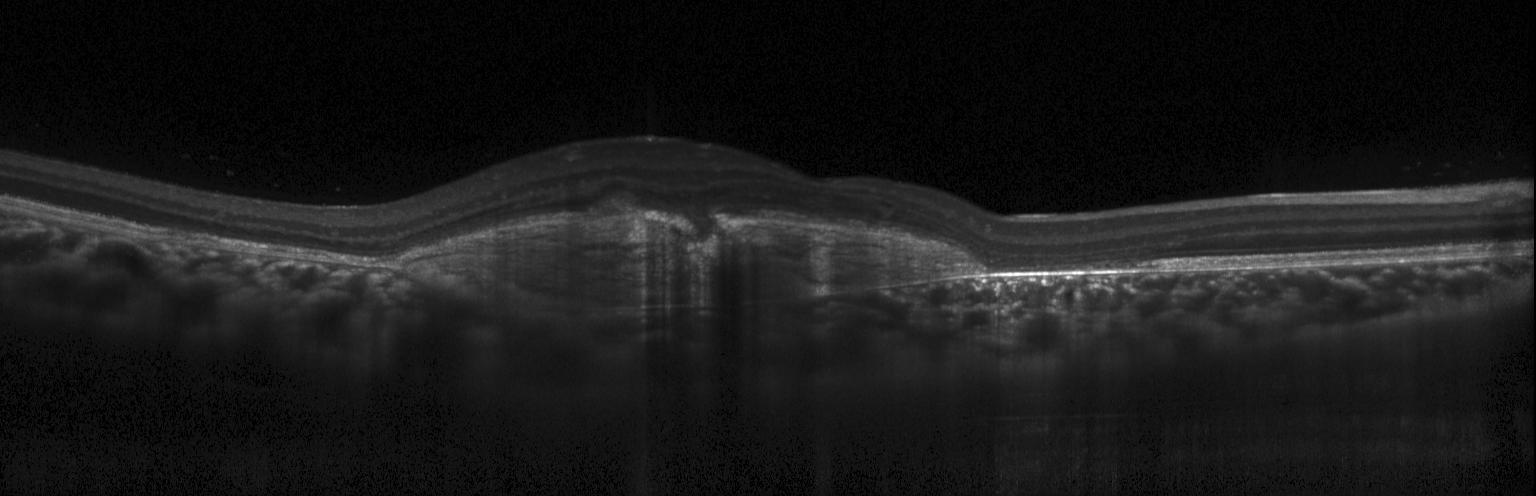

OCT scan showing a choroidal neovascular membrane.